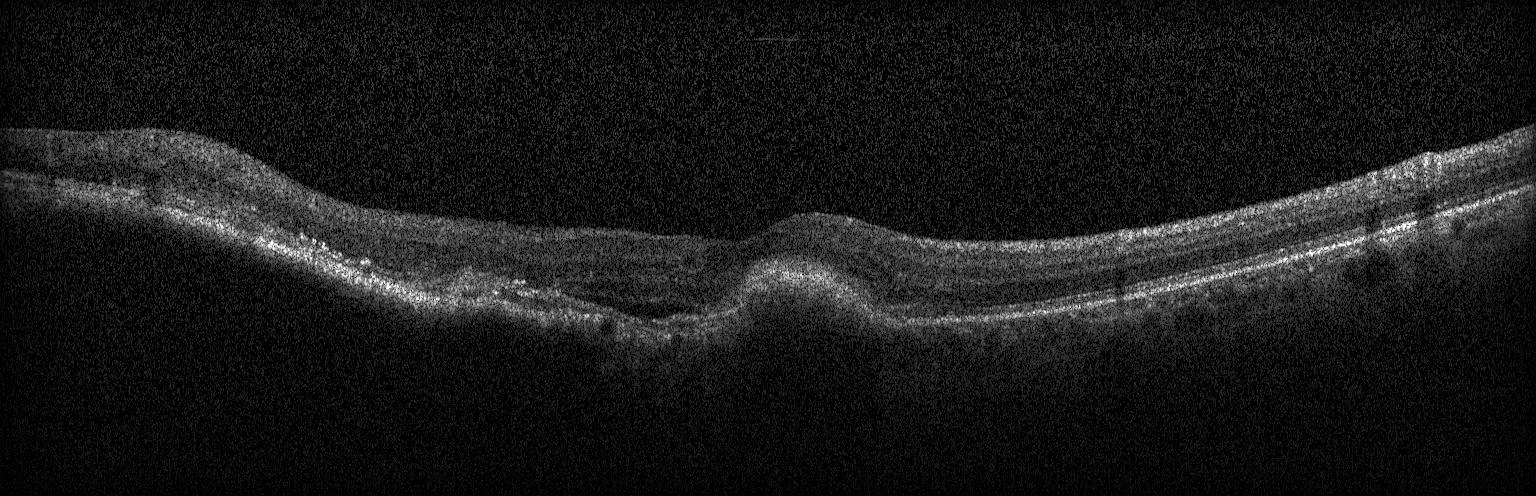
Heidelberg Spectralis OCT system. Horizontal scan through the fovea. Retinal OCT cross-section.
Finding: a choroidal neovascular membrane.